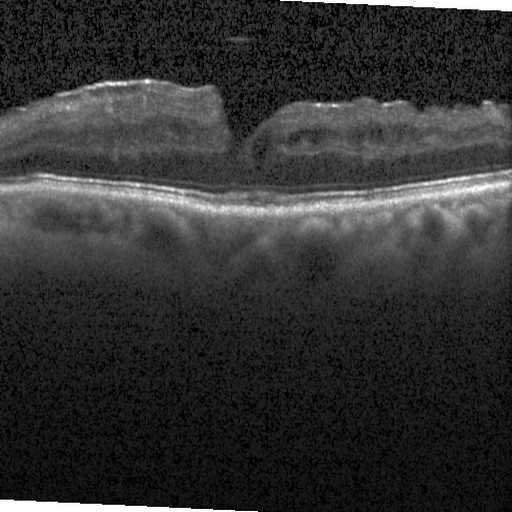

Fovea-centered, optical coherence tomography B-scan, instrument: Heidelberg Spectralis, spectral-domain optical coherence tomography. Diagnosis: diabetic macular edema (DME).